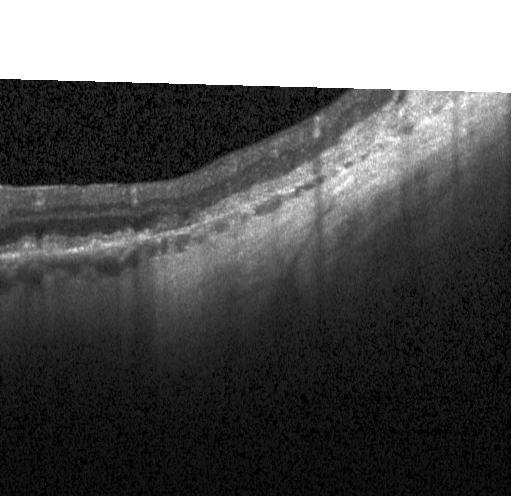

Retinal OCT cross-section
This B-scan demonstrates choroidal neovascularization.